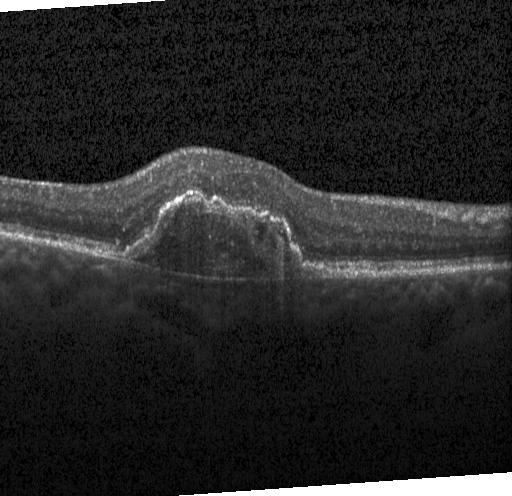

This B-scan demonstrates choroidal neovascularization.